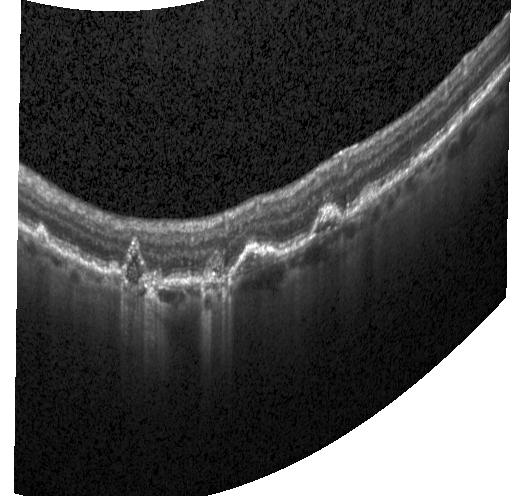
Diagnosis: a choroidal neovascular membrane.